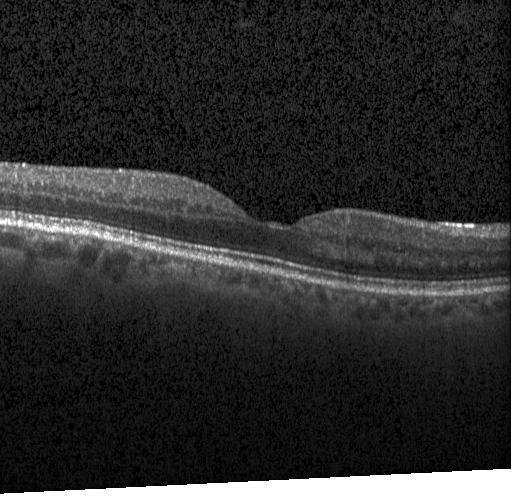
Optical coherence tomography scan — Impression: neither choroidal neovascularization, diabetic macular edema, nor drusen.